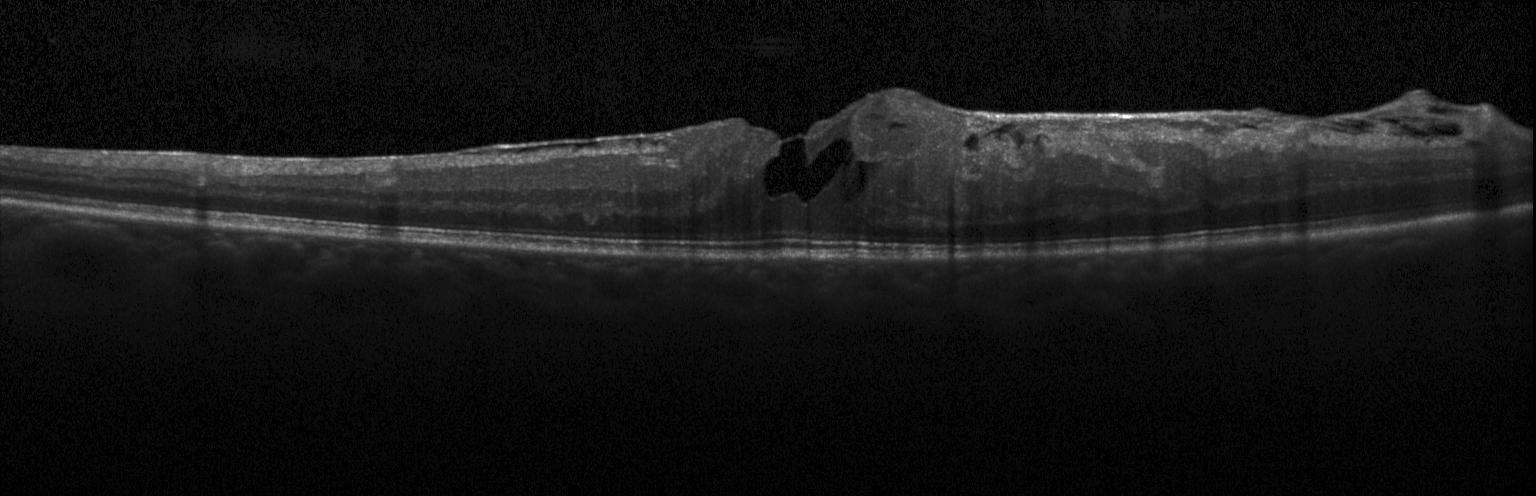 Finding: diabetic macular edema (DME).